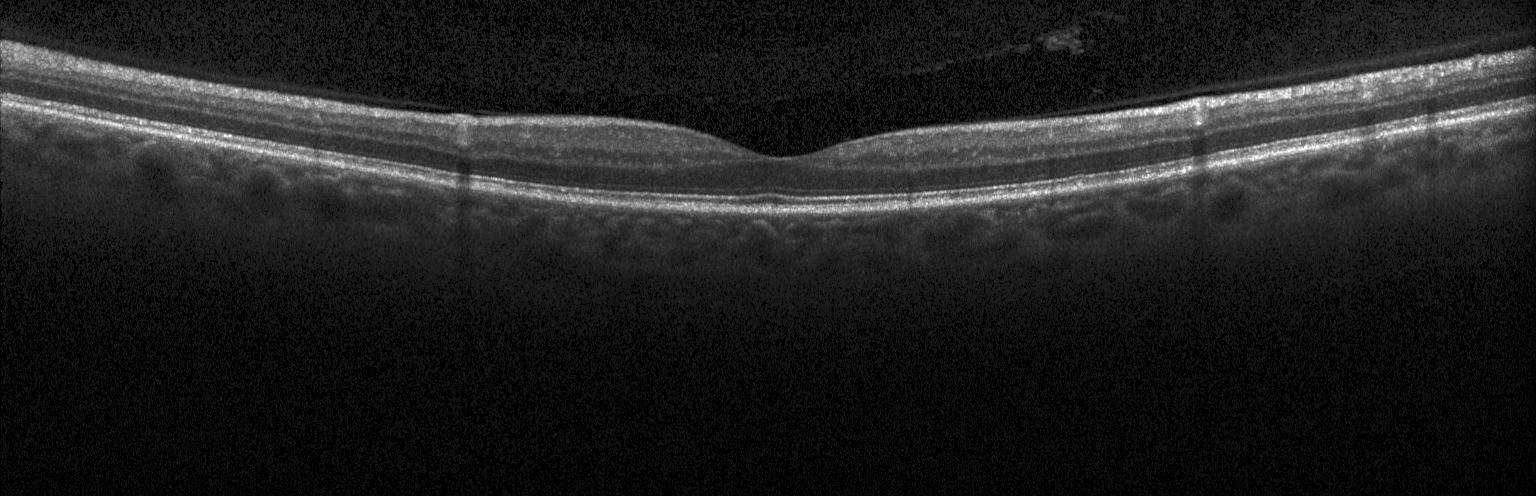
Retinal OCT cross-section; horizontal scan through the fovea — Assessment: neither choroidal neovascularization, diabetic macular edema, nor drusen.